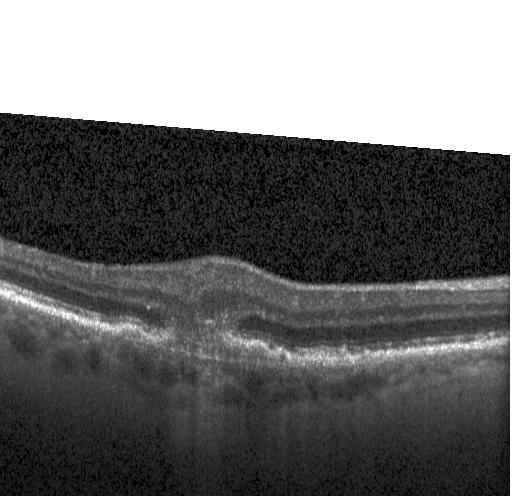
SD-OCT, Heidelberg Spectralis, OCT B-scan — Macular OCT: a choroidal neovascular membrane.